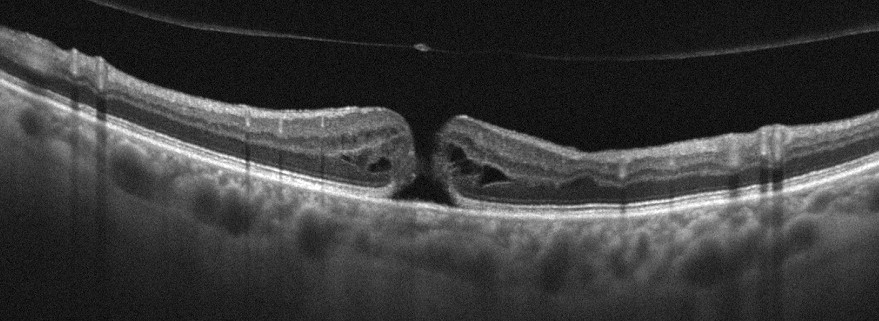
Fovea-centered. Retinal OCT cross-section. Optovue Avanti RTVue XR
Macular OCT: vitreomacular interface disease (VID).